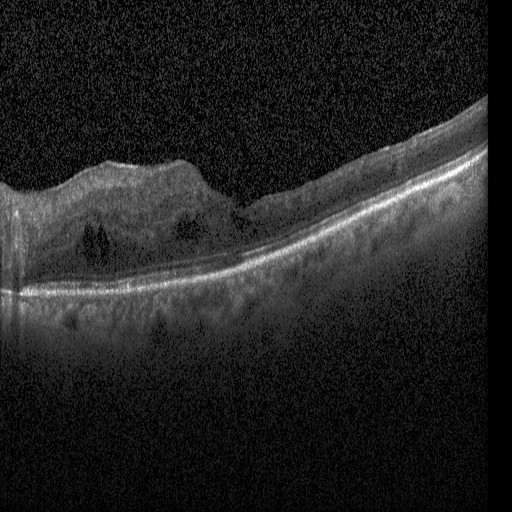
Retinal OCT B-scan, macular scan — Impression: DME.